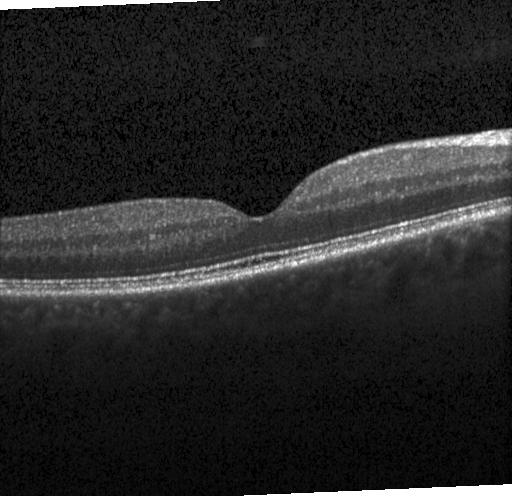
Retinal OCT cross-section · spectral-domain optical coherence tomography
Impression: no evidence of choroidal neovascularization, diabetic macular edema, or drusen.